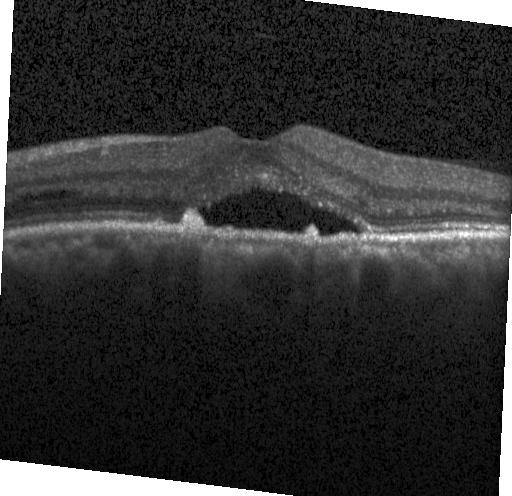

Heidelberg Spectralis OCT system. Optical coherence tomography B-scan. Fovea-centered. Spectral-domain OCT.
OCT finding: a choroidal neovascular membrane.